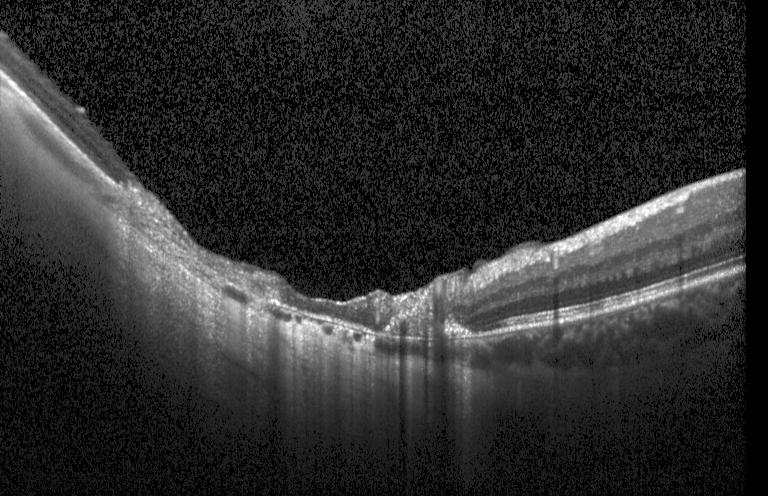

Heidelberg Spectralis OCT system; fovea-centered; retinal OCT B-scan; spectral-domain optical coherence tomography — Impression: a choroidal neovascular membrane.